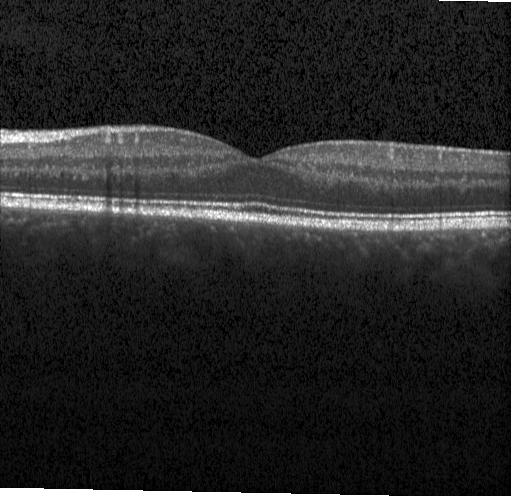 Acquired on a Heidelberg Spectralis; optical coherence tomography scan. Diagnosis: no CNV, no DME, and no drusen.